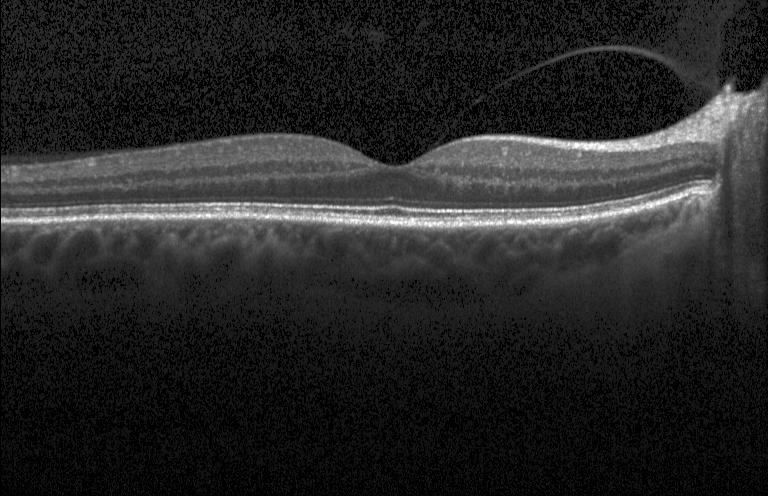
Retinal OCT cross-section showing no choroidal neovascularization, diabetic macular edema, or drusen.